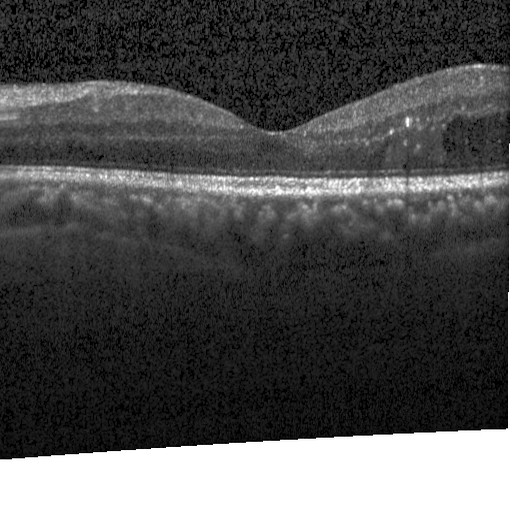
Macular OCT: diabetic macular edema.